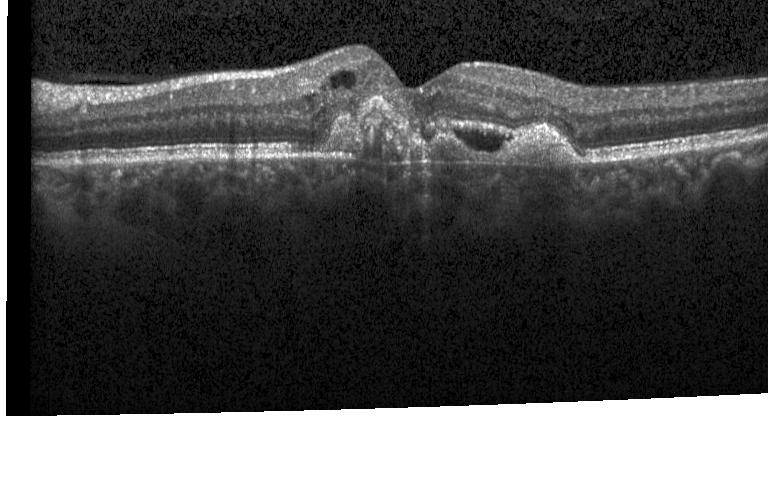 A choroidal neovascular membrane.